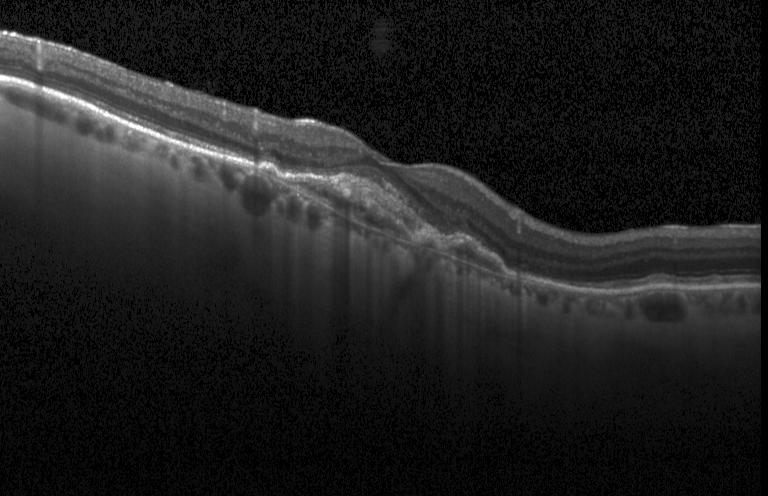
Optical coherence tomography B-scan.
Impression: a choroidal neovascular membrane.